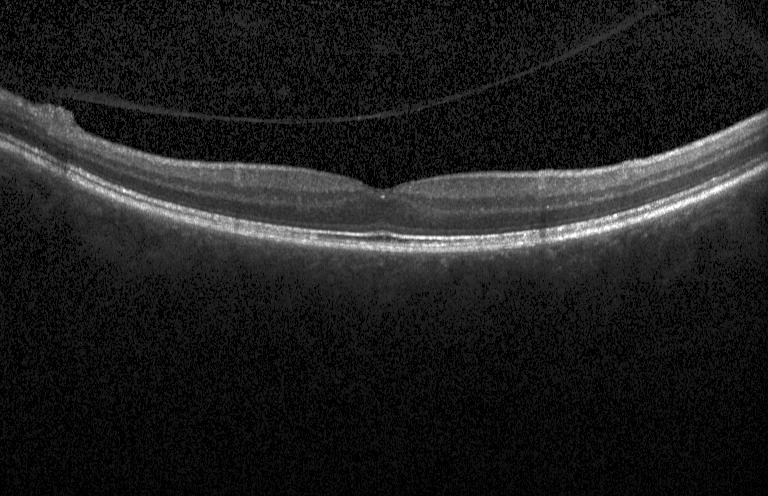 Assessment: no CNV, no DME, and no drusen.